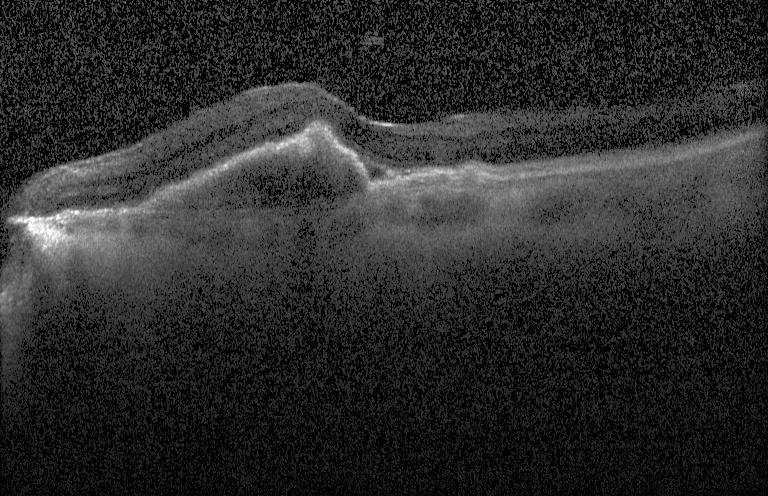
Macular OCT: a choroidal neovascular membrane.